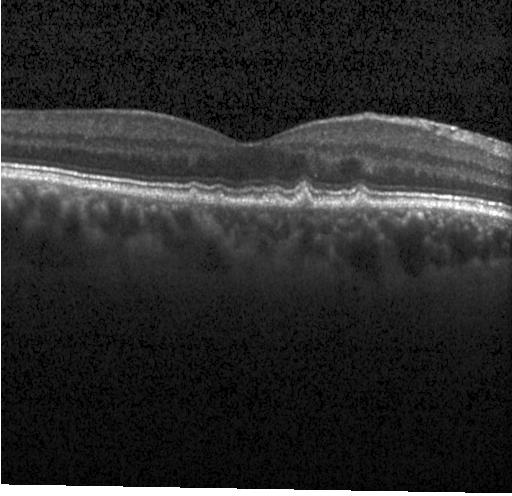 Acquired on a Heidelberg Spectralis; retinal OCT cross-section; spectral-domain optical coherence tomography — Macular OCT: multiple drusen.